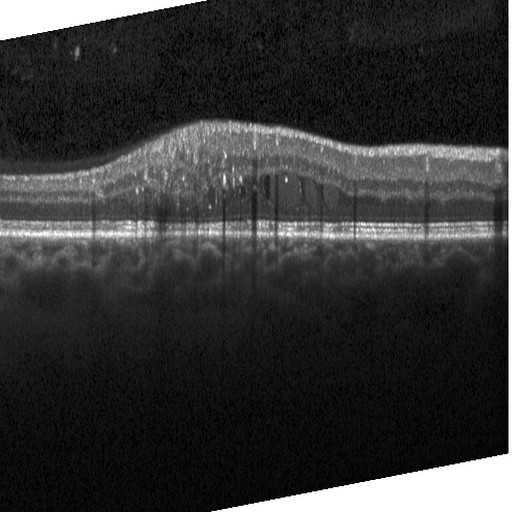

OCT B-scan, fovea-centered, SD-OCT.
Diagnosis: DME.